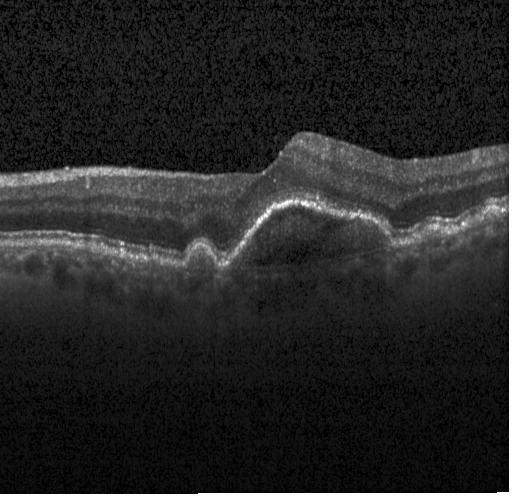
Optical coherence tomography scan
Sub-RPE drusenoid deposits.